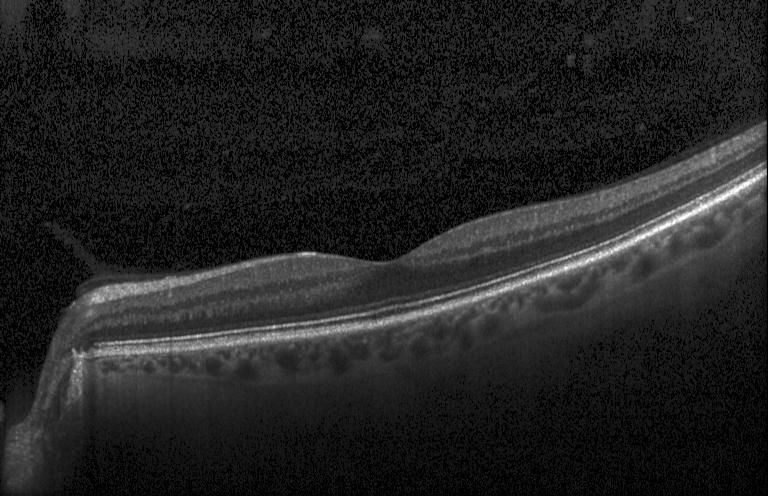

OCT line scan
Dx: neither choroidal neovascularization, diabetic macular edema, nor drusen.